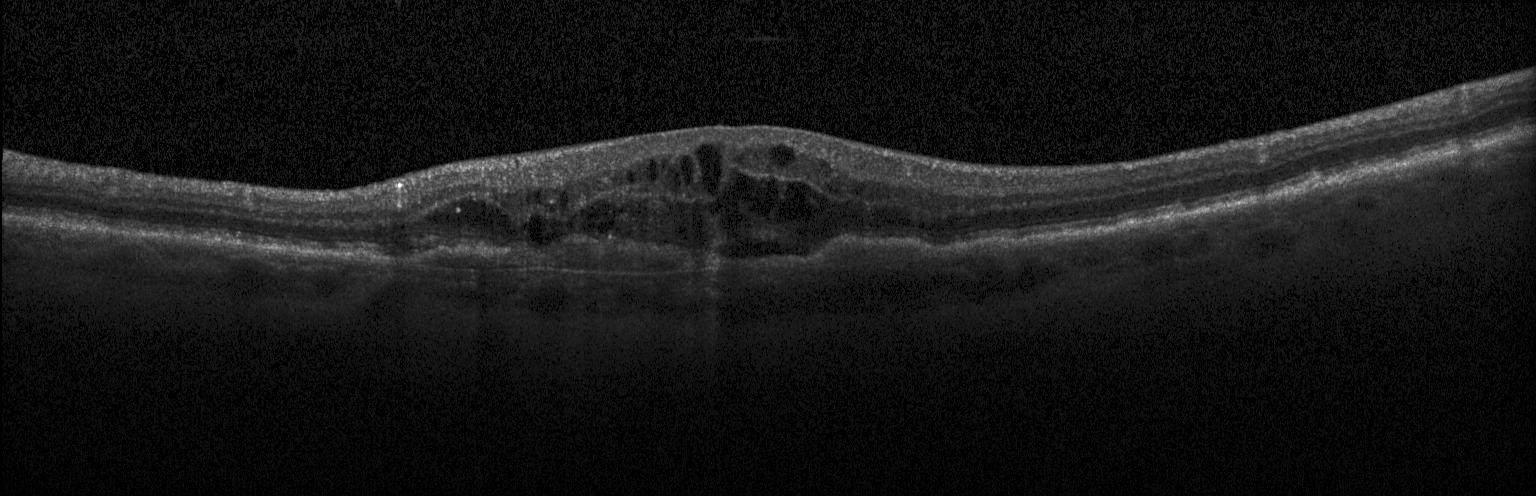 Retinal OCT B-scan · Heidelberg Spectralis · fovea-centered · spectral-domain OCT. Diagnosis: a choroidal neovascular membrane.